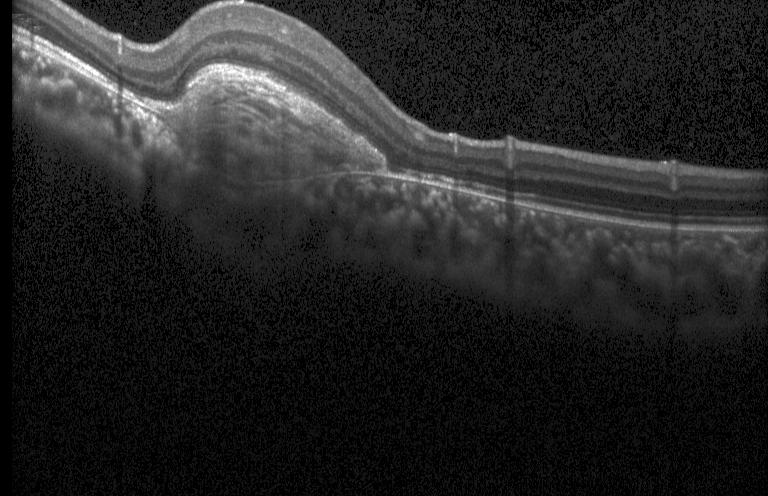 Horizontal scan through the fovea · retinal OCT cross-section.
Dx: a choroidal neovascular membrane.